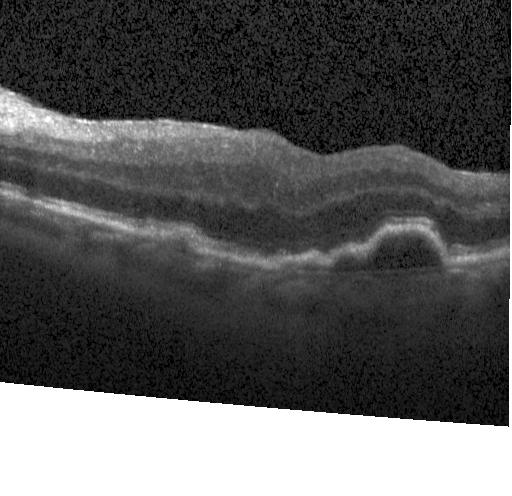

SD-OCT · OCT B-scan · macular scan. Assessment: a choroidal neovascular membrane.